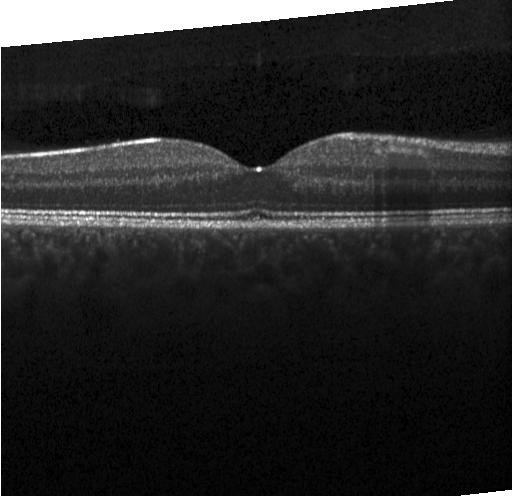

Finding: no evidence of choroidal neovascularization, diabetic macular edema, or drusen.